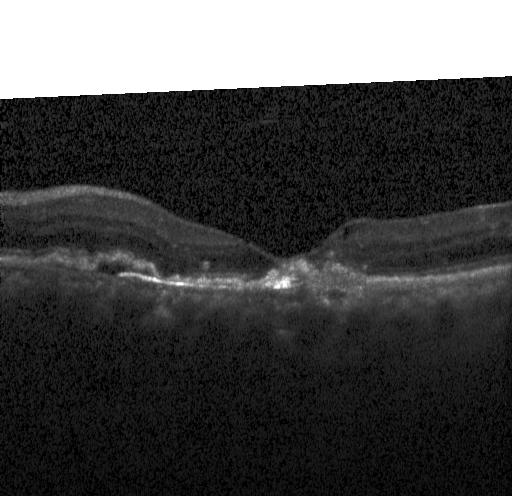 OCT line scan — A choroidal neovascular membrane.